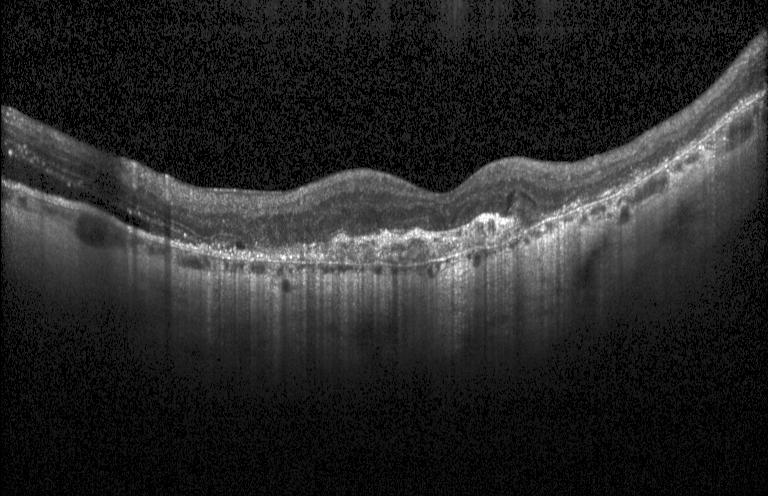 Assessment: a choroidal neovascular membrane.